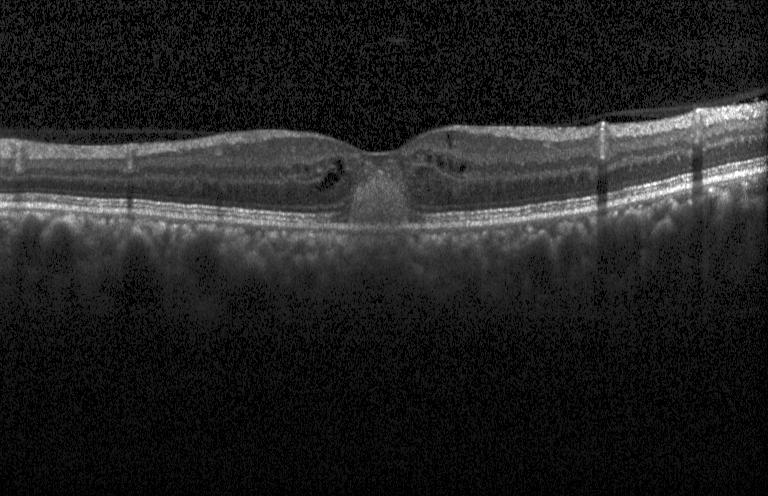
Finding: a choroidal neovascular membrane.